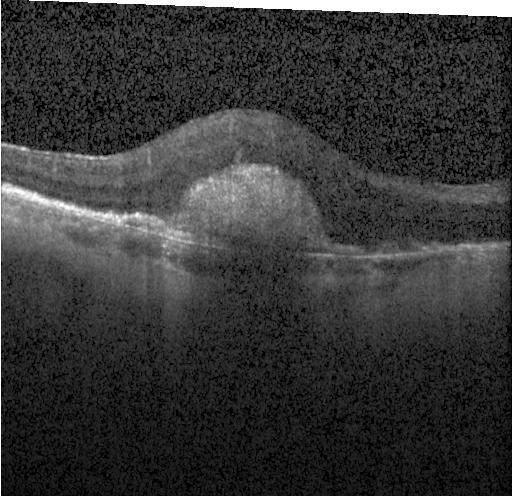
Heidelberg Spectralis, optical coherence tomography scan.
Finding: choroidal neovascularization (CNV).